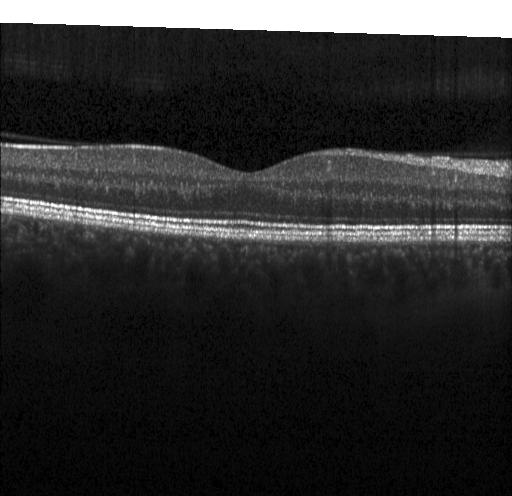 OCT finding: no CNV, no DME, and no drusen.